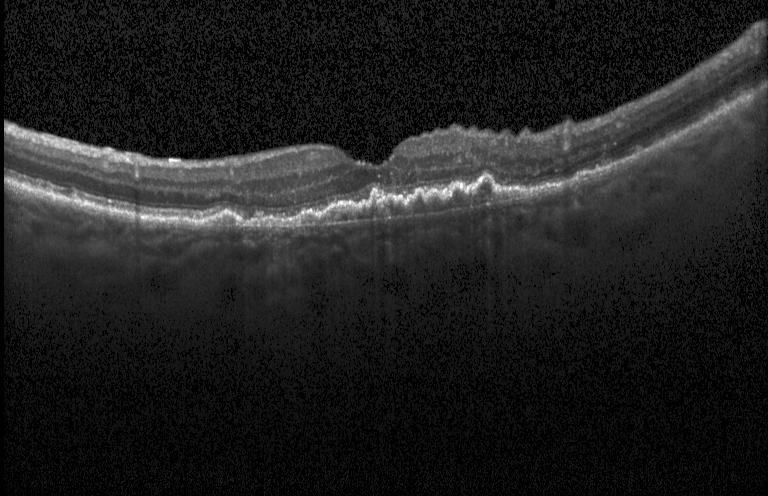

Retinal OCT cross-section · fovea-centered — Impression: a choroidal neovascular membrane.